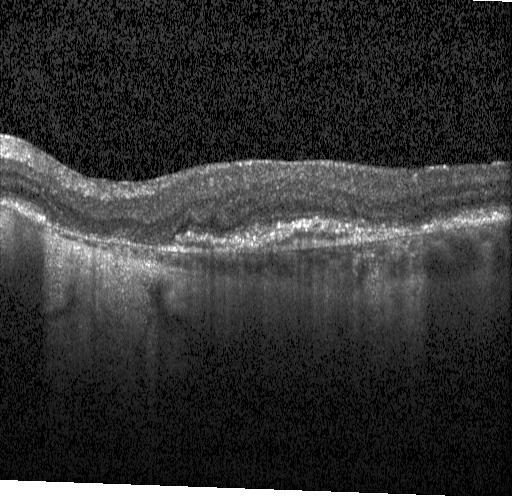
Finding: a choroidal neovascular membrane.